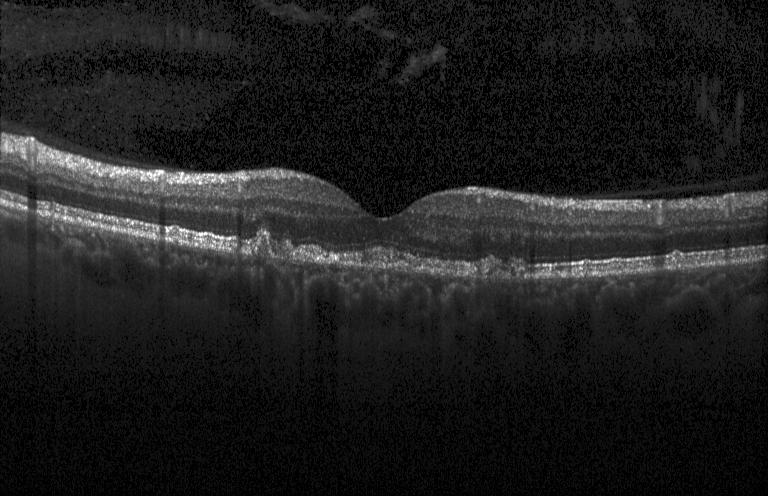

Spectral-domain optical coherence tomography · optical coherence tomography B-scan. Assessment: drusen.